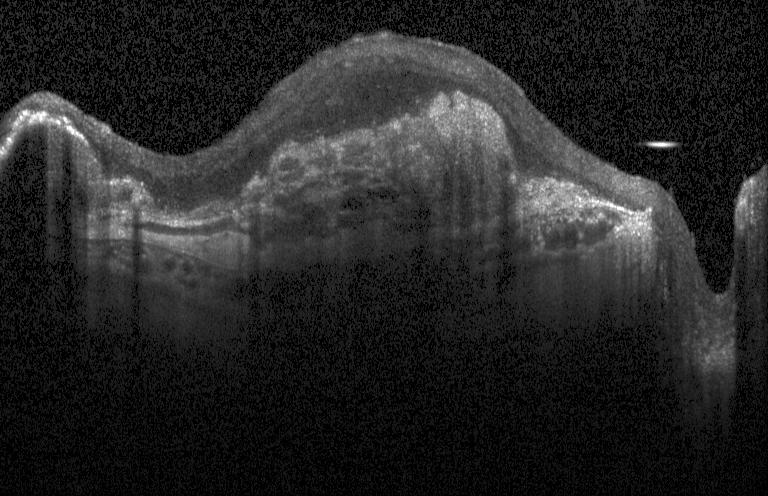

Spectral-domain OCT · optical coherence tomography B-scan.
Impression: a choroidal neovascular membrane.